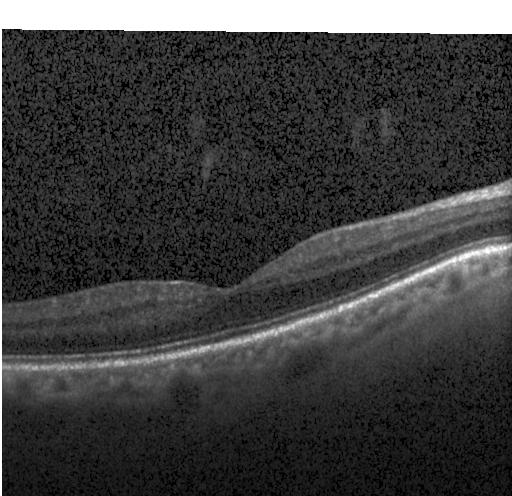
Diagnosis: no choroidal neovascularization, no diabetic macular edema, and no drusen.